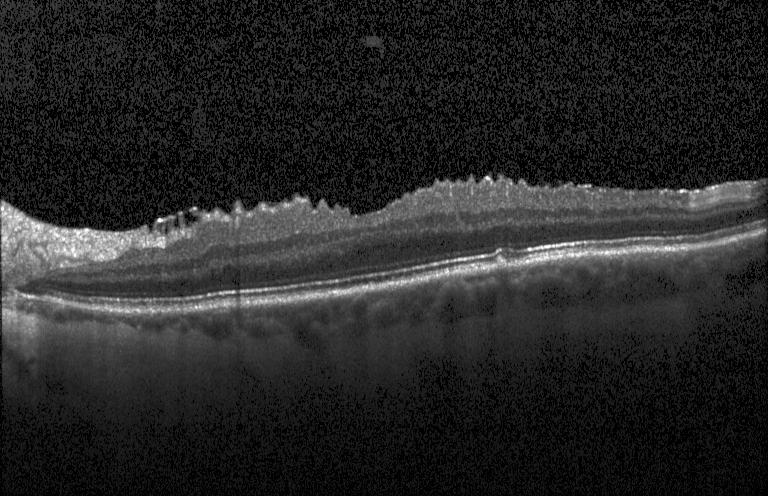

Macular OCT: sub-RPE drusenoid deposits.